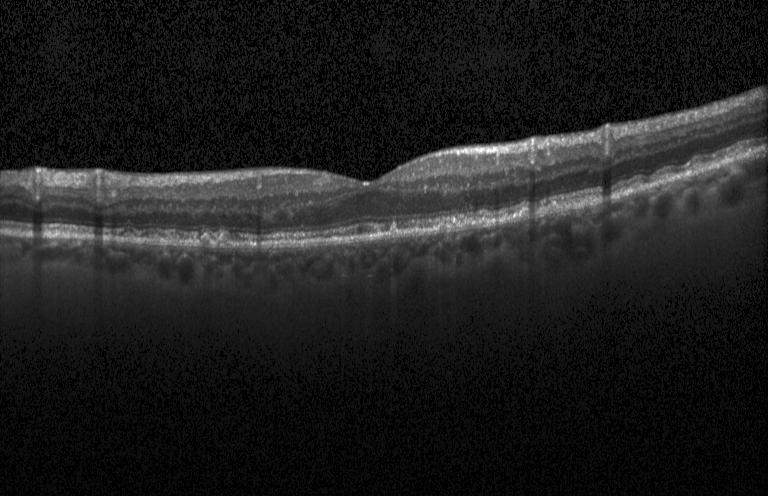 Macular OCT: drusen.